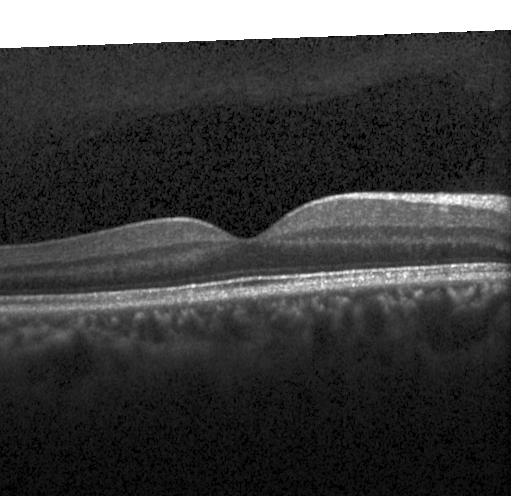
Spectral-domain optical coherence tomography. Instrument: Heidelberg Spectralis. Through the macula. OCT B-scan. Impression: no evidence of choroidal neovascularization, diabetic macular edema, or drusen.